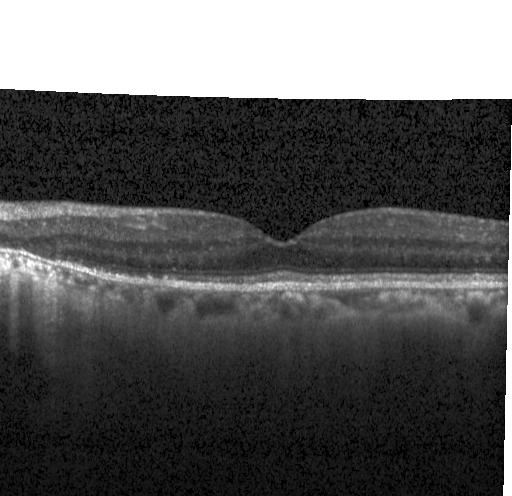 Finding: neither choroidal neovascularization, diabetic macular edema, nor drusen.